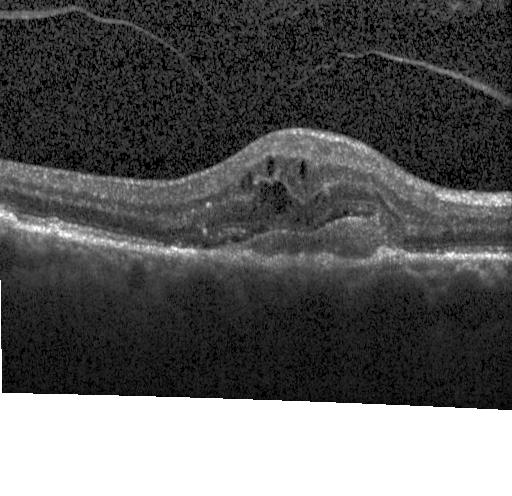
Diagnosis: CNV.